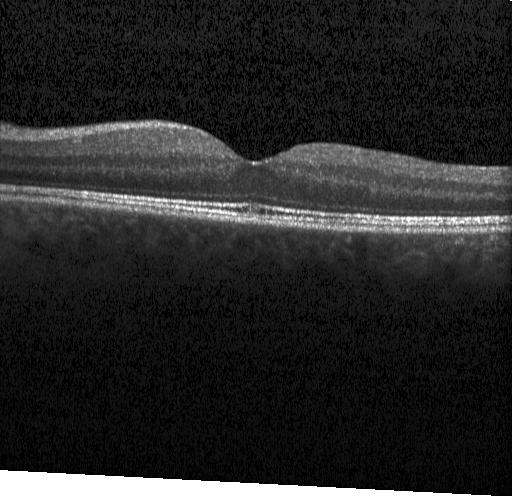
Retinal OCT cross-section
Impression: no CNV, DME, or drusen.